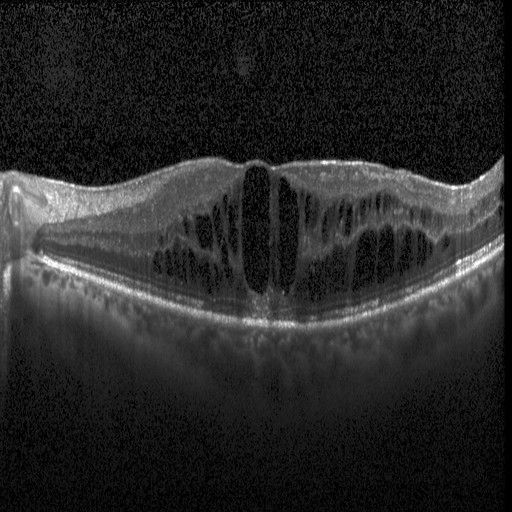 Optical coherence tomography B-scan. SD-OCT. Macular scan. Heidelberg Spectralis OCT system. Diabetic macular edema.